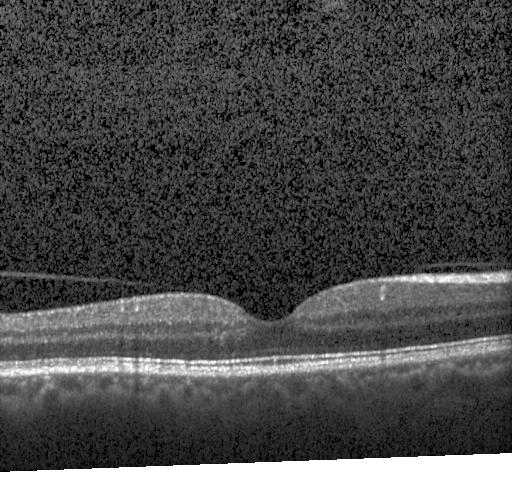 OCT finding: no evidence of CNV, DME, or drusen.